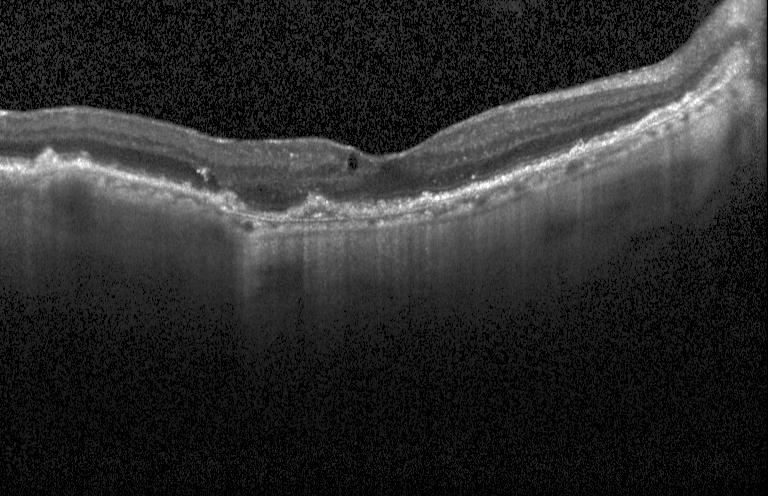

OCT line scan. Acquired on a Heidelberg Spectralis. Finding: a choroidal neovascular membrane.